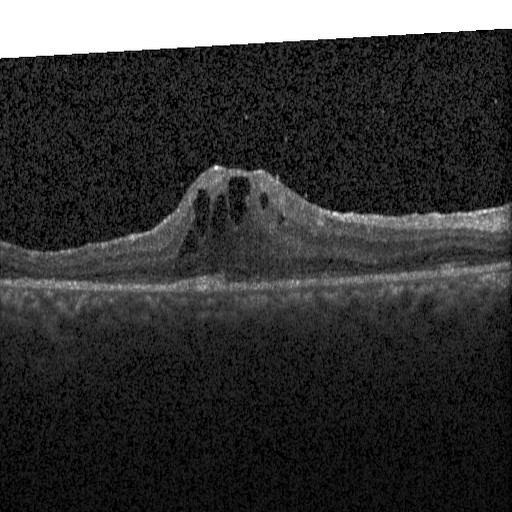
Retinal OCT B-scan; horizontal scan through the fovea; SD-OCT; Heidelberg Spectralis — Assessment: diabetic macular edema.